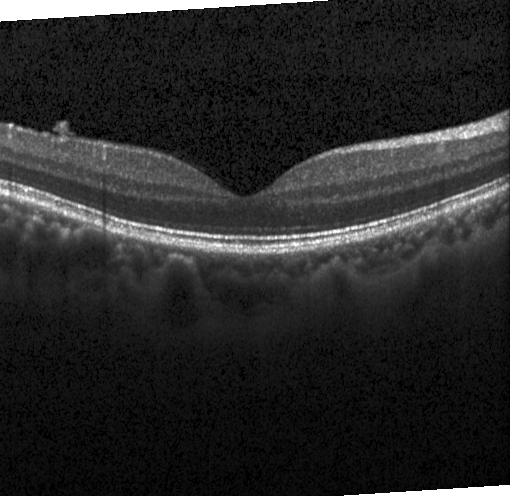 Heidelberg Spectralis OCT system · OCT line scan — Diagnosis: no choroidal neovascularization, diabetic macular edema, or drusen.